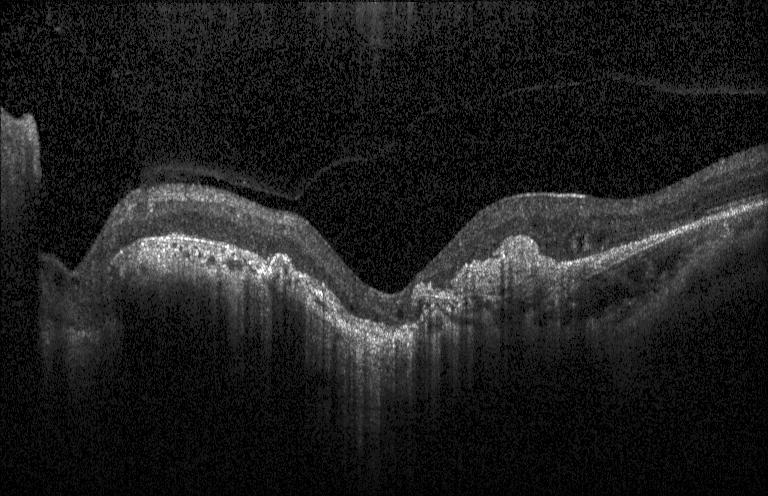 This B-scan demonstrates choroidal neovascularization.